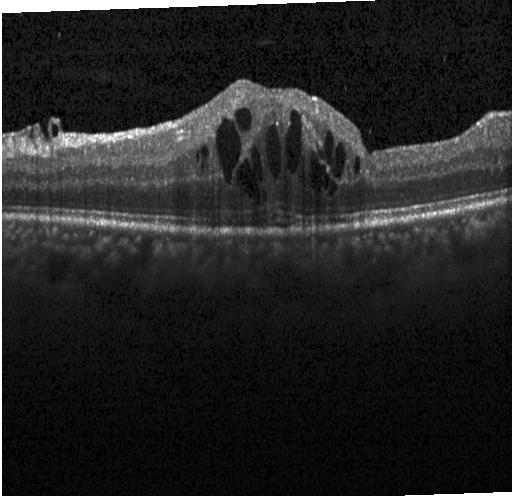 Retinal OCT cross-section; macular scan; spectral-domain OCT; acquired on a Heidelberg Spectralis
Impression: DME.